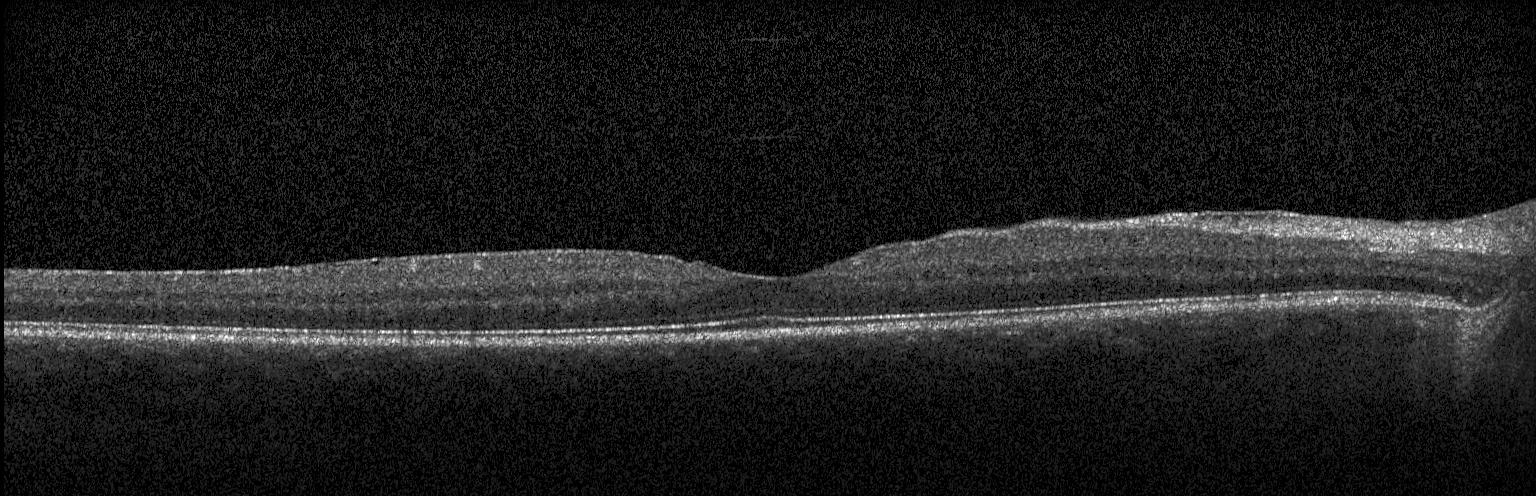
Optical coherence tomography B-scan — OCT finding: no evidence of choroidal neovascularization, diabetic macular edema, or drusen.